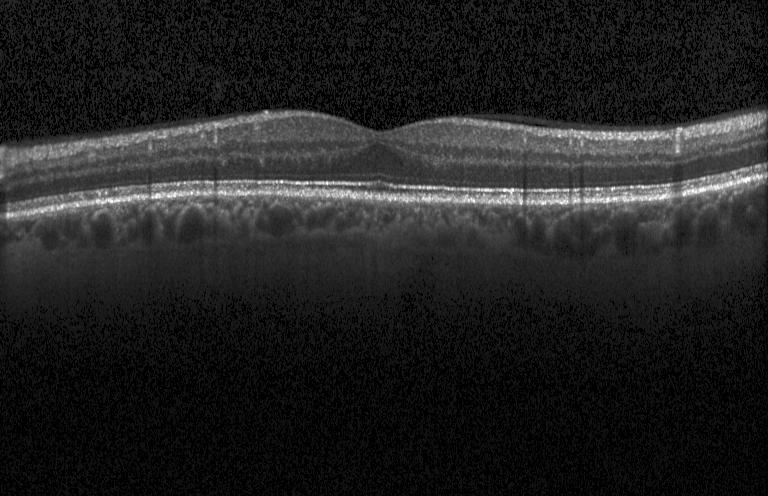
OCT B-scan showing no choroidal neovascularization, diabetic macular edema, or drusen.